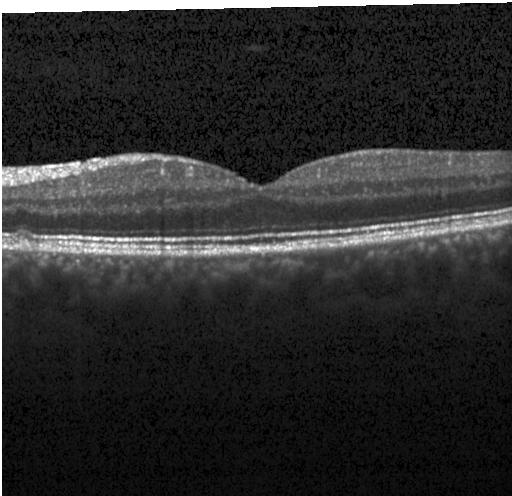 Retinal OCT cross-section, through the macula, spectral-domain optical coherence tomography, Heidelberg Spectralis OCT system
OCT finding: multiple drusen.